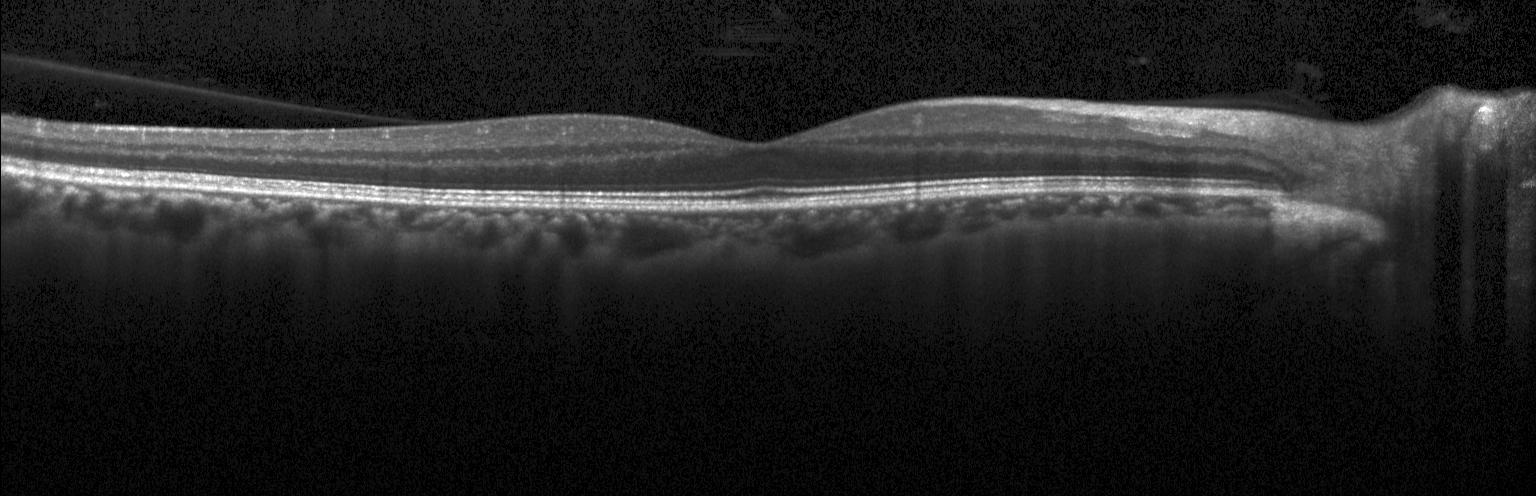
SD-OCT, instrument: Heidelberg Spectralis, retinal OCT cross-section, macular scan — Dx: neither choroidal neovascularization, diabetic macular edema, nor drusen.